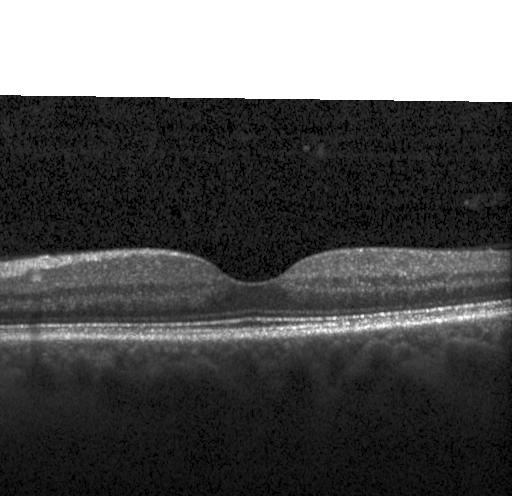 Optical coherence tomography scan. Neither CNV, DME, nor drusen.